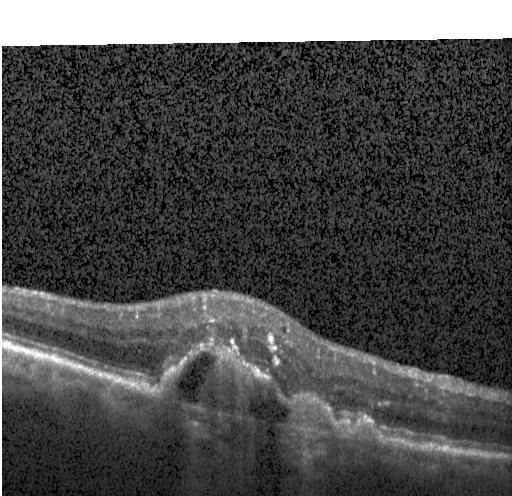 Spectral-domain OCT B-scan: a choroidal neovascular membrane.